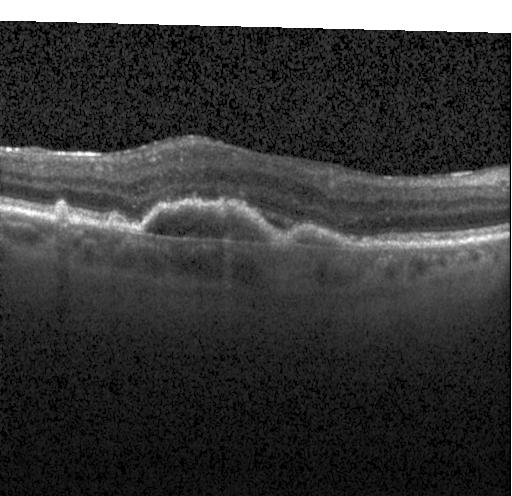

Through the macula · OCT line scan · spectral-domain optical coherence tomography
Impression: CNV.